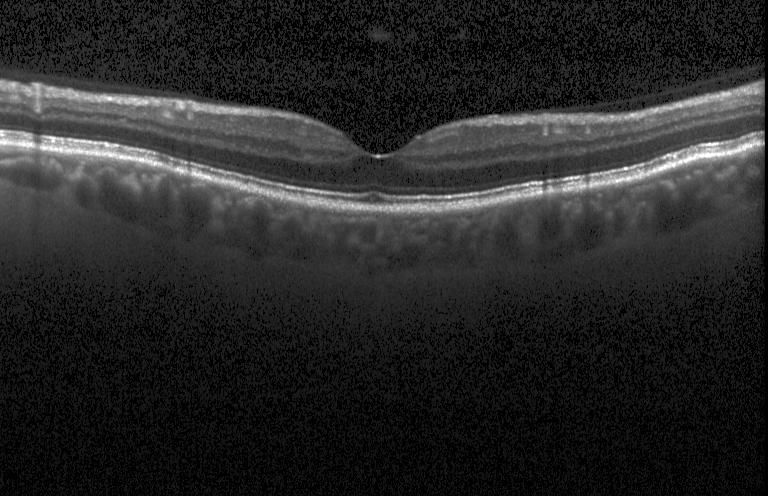
Dx: no choroidal neovascularization, no diabetic macular edema, and no drusen.